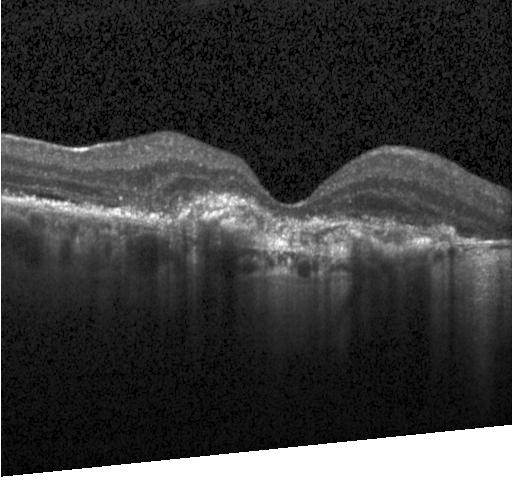

Heidelberg Spectralis; OCT line scan; centered on the fovea; spectral-domain optical coherence tomography. Diagnosis: a choroidal neovascular membrane.